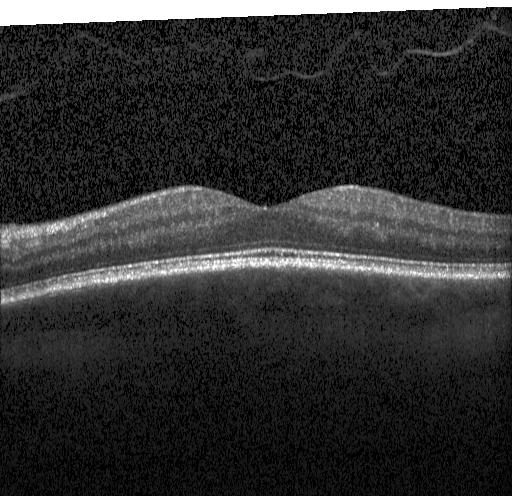

Neither choroidal neovascularization, diabetic macular edema, nor drusen.